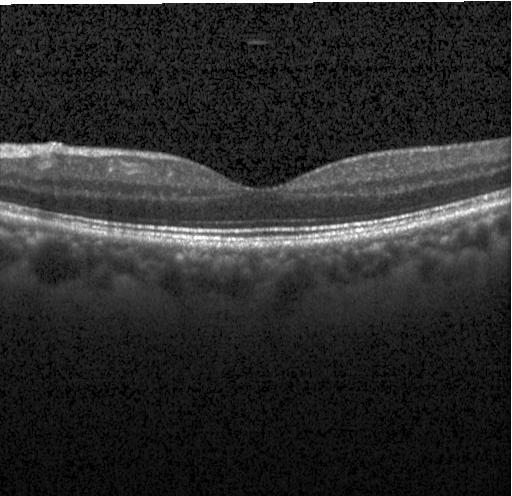

Spectral-domain OCT B-scan: neither choroidal neovascularization, diabetic macular edema, nor drusen.